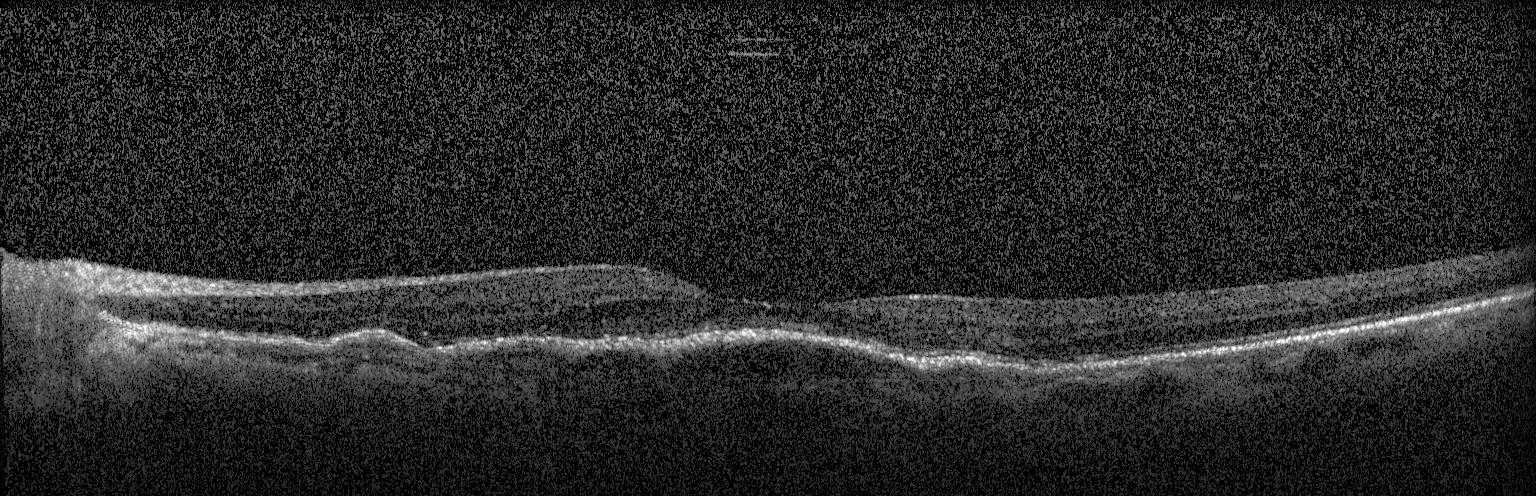

Diagnosis: a choroidal neovascular membrane.